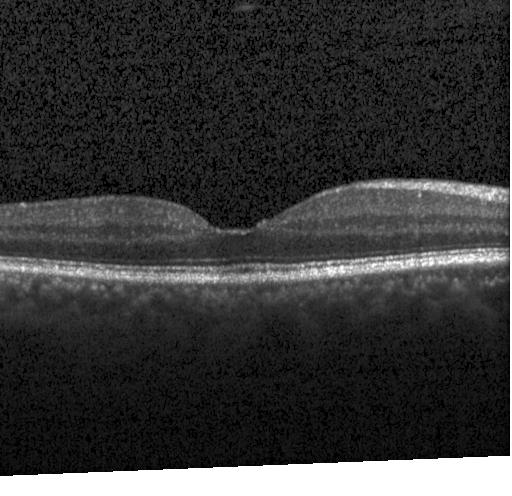
Optical coherence tomography scan.
Diagnosis: no CNV, DME, or drusen.